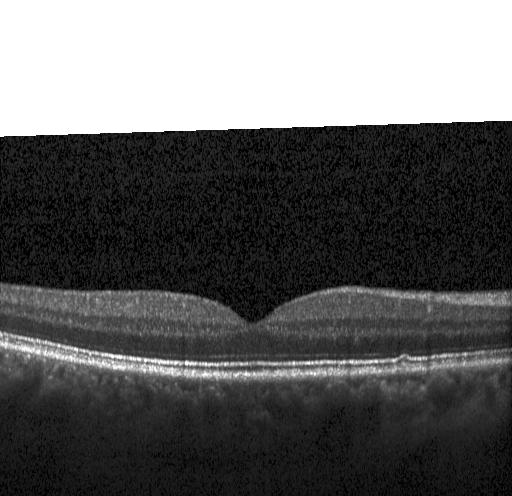
Retinal OCT cross-section, horizontal scan through the fovea
Diagnosis: drusen.